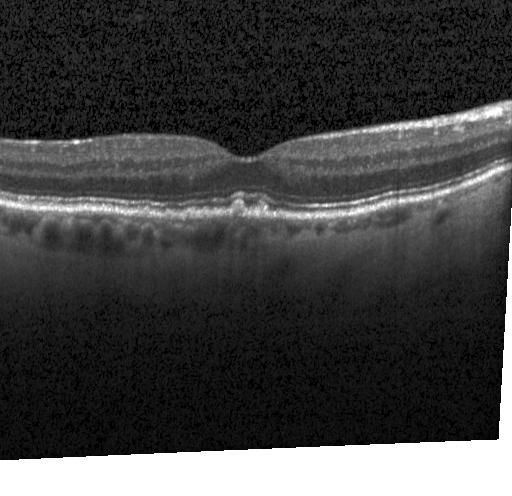

Retinal OCT cross-section — The scan shows drusen.